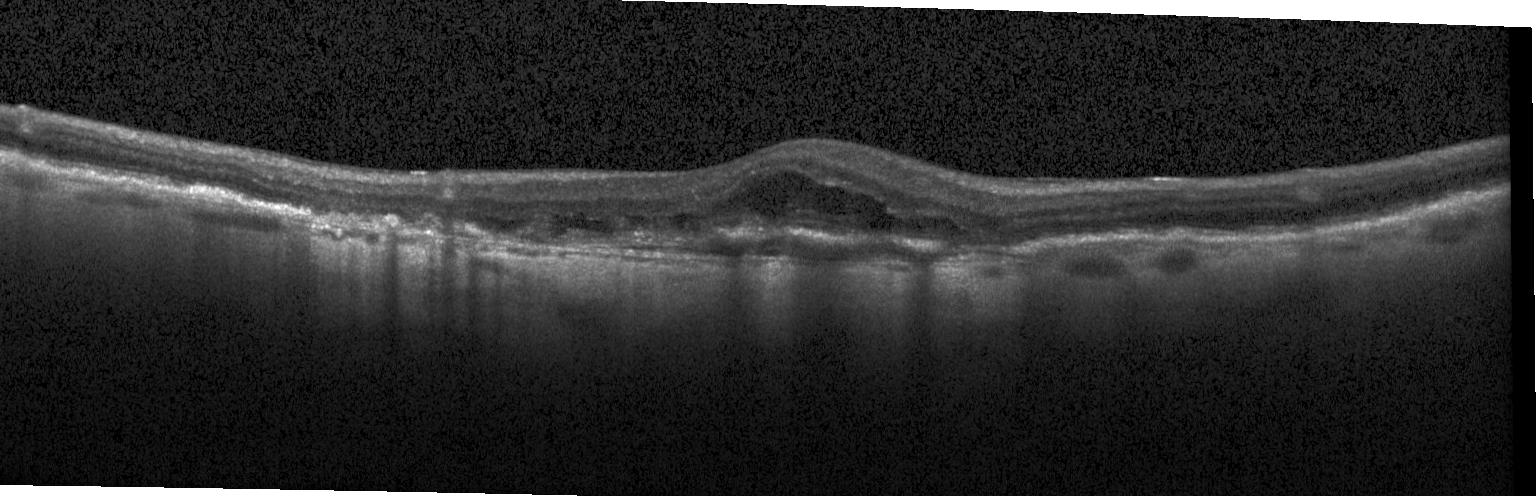
Retinal OCT cross-section · Heidelberg Spectralis OCT system · through the macula · SD-OCT
This B-scan demonstrates a choroidal neovascular membrane.